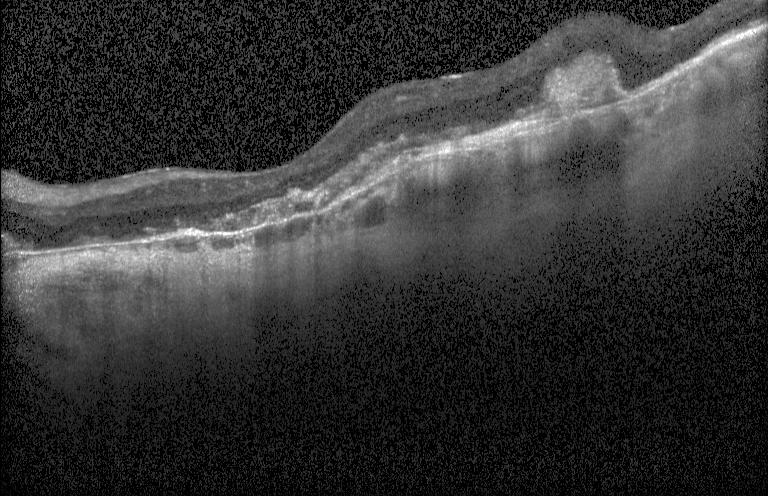

OCT line scan.
Diagnosis: CNV.